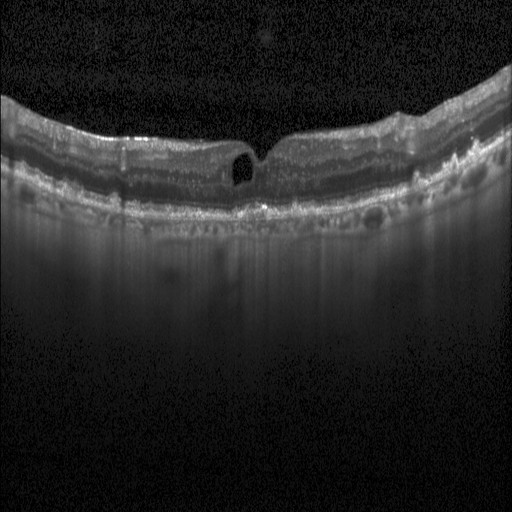

Heidelberg Spectralis OCT system, retinal OCT cross-section, macular scan
Diagnosis: diabetic macular edema (DME).